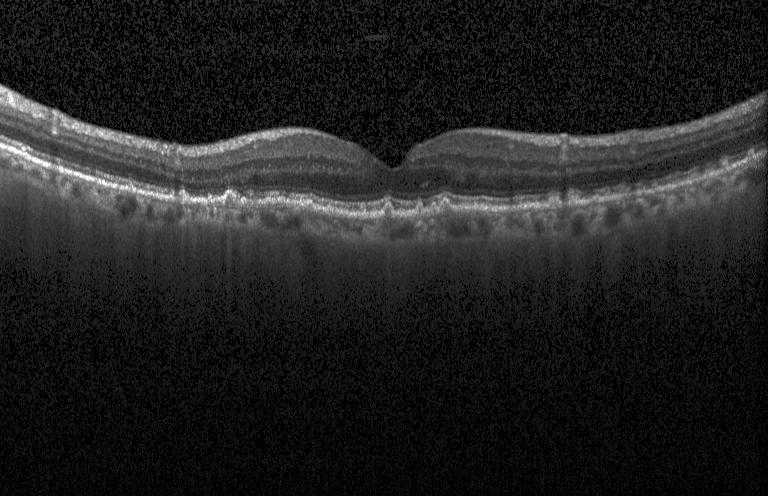 Acquired on a Heidelberg Spectralis · retinal OCT B-scan · horizontal scan through the fovea · SD-OCT — Diagnosis: multiple drusen.